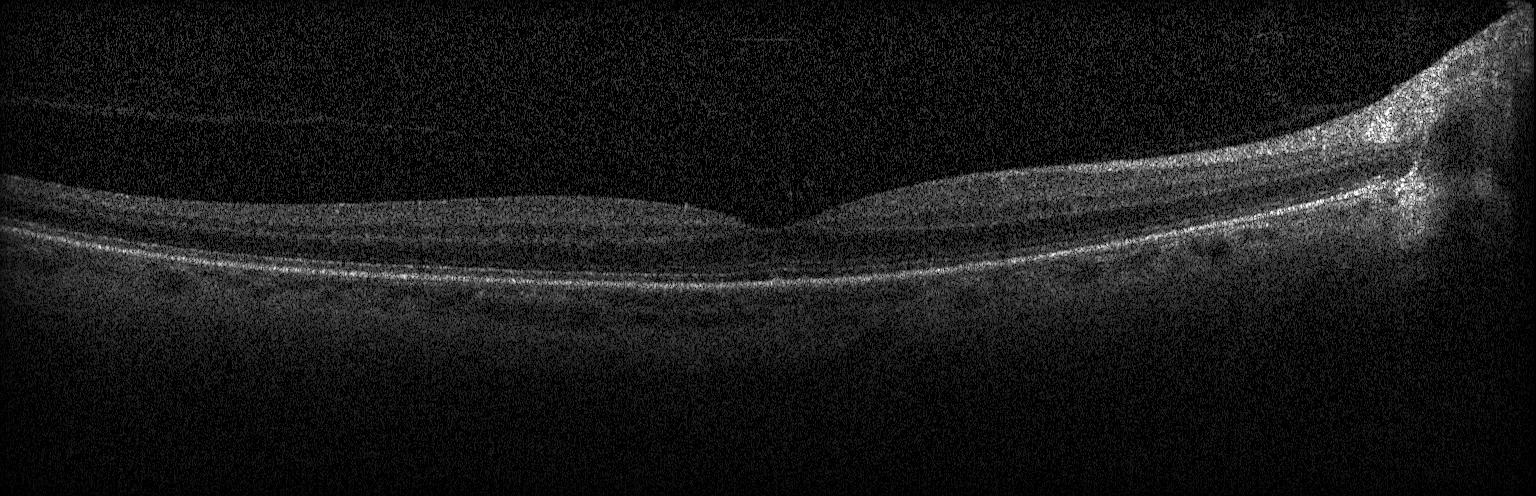 OCT line scan; horizontal scan through the fovea.
Assessment: no choroidal neovascularization, diabetic macular edema, or drusen.